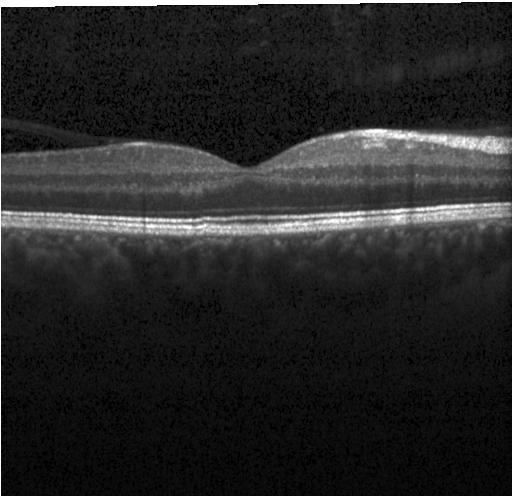
Macular scan. Spectral-domain OCT. OCT B-scan. Instrument: Heidelberg Spectralis. No evidence of CNV, DME, or drusen.